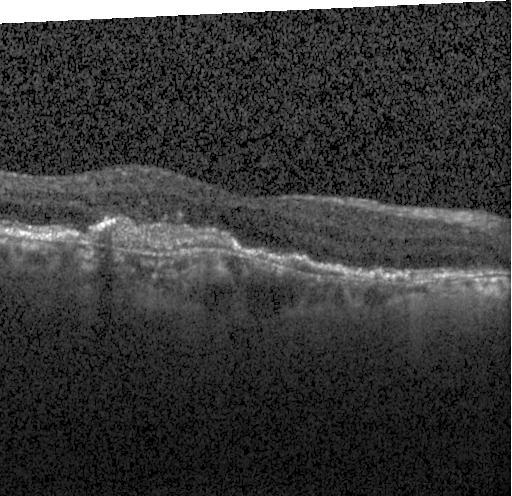 Diagnosis: a choroidal neovascular membrane.